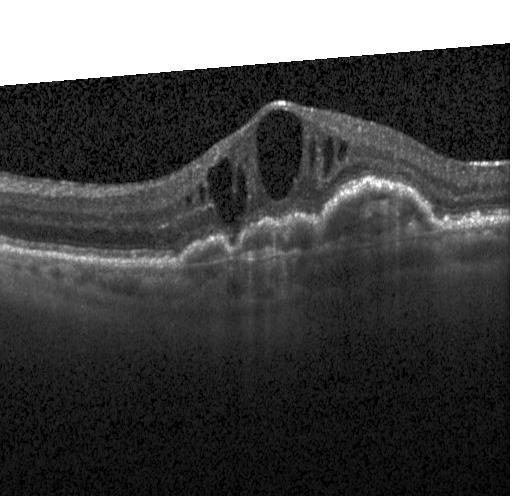
Diagnosis: choroidal neovascularization.